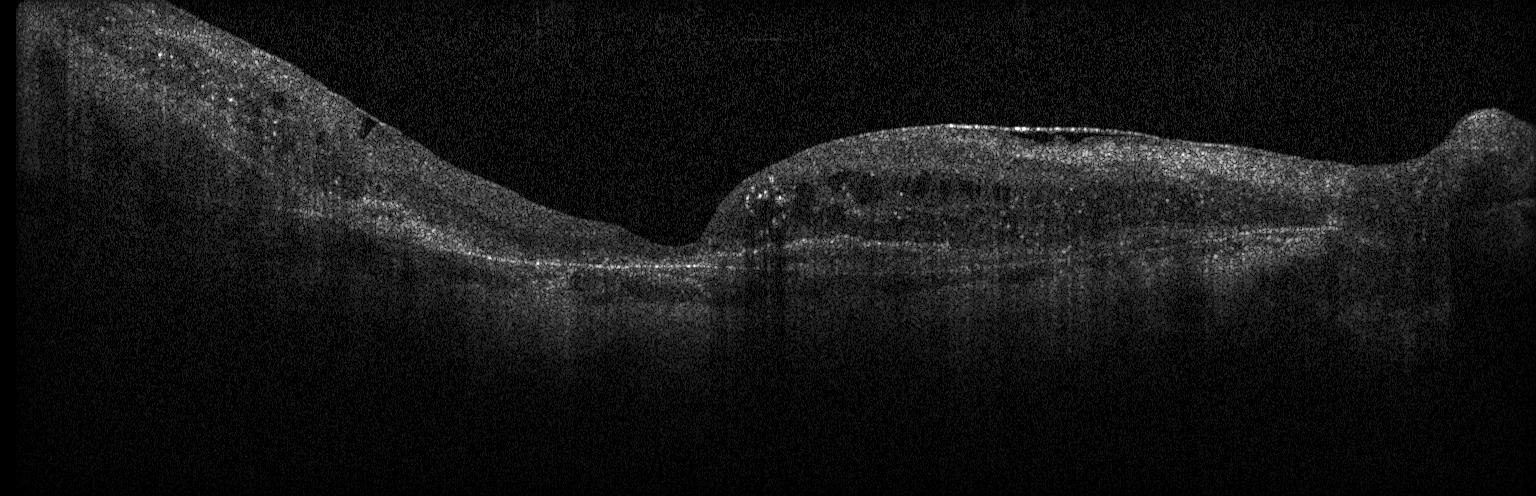
OCT line scan; through the macula.
Diagnosis: CNV.